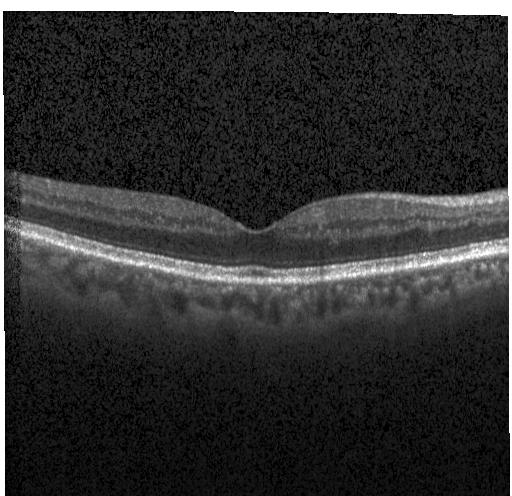

OCT line scan. Finding: no choroidal neovascularization, no diabetic macular edema, and no drusen.